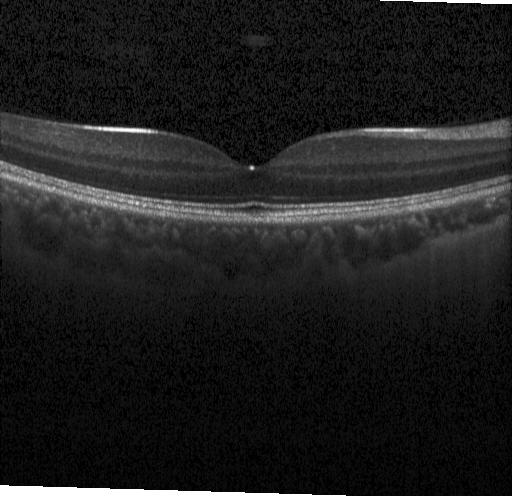

Optical coherence tomography B-scan, SD-OCT
No choroidal neovascularization, diabetic macular edema, or drusen.